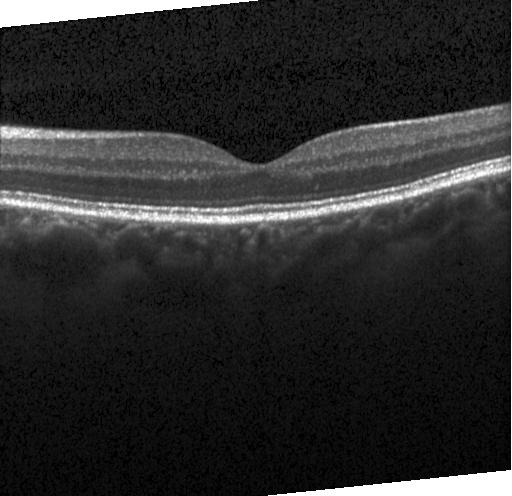

Centered on the fovea, instrument: Heidelberg Spectralis, OCT line scan. Finding: no CNV, no DME, and no drusen.